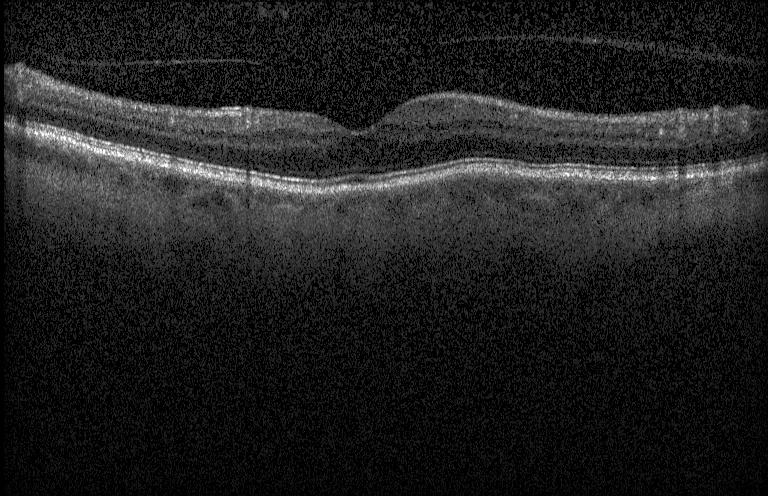
No evidence of choroidal neovascularization, diabetic macular edema, or drusen.